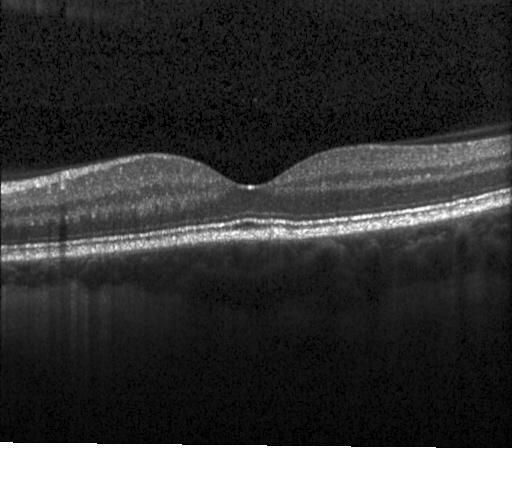

Finding: no evidence of choroidal neovascularization, diabetic macular edema, or drusen.